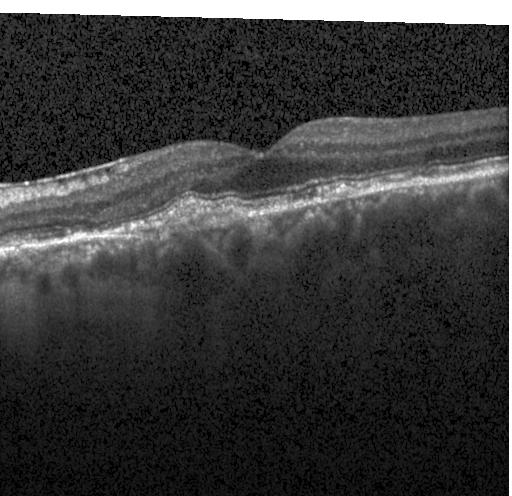
Heidelberg Spectralis; spectral-domain optical coherence tomography; retinal OCT cross-section; macular scan.
Macular OCT: a choroidal neovascular membrane.